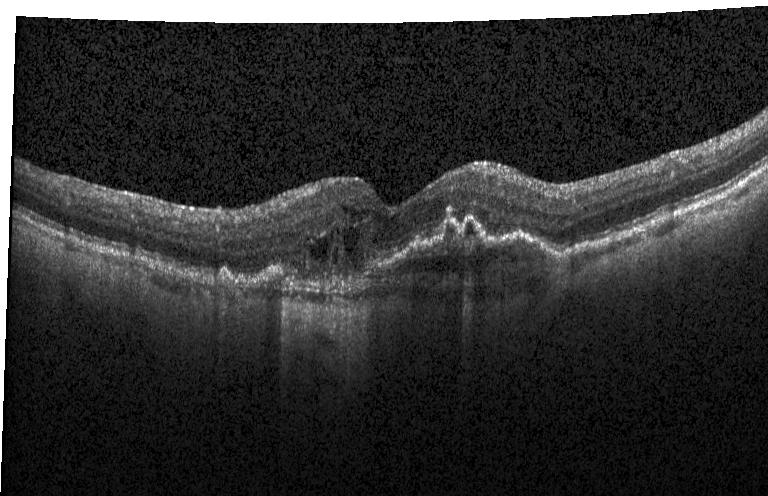

Retinal OCT B-scan. Assessment: choroidal neovascularization.